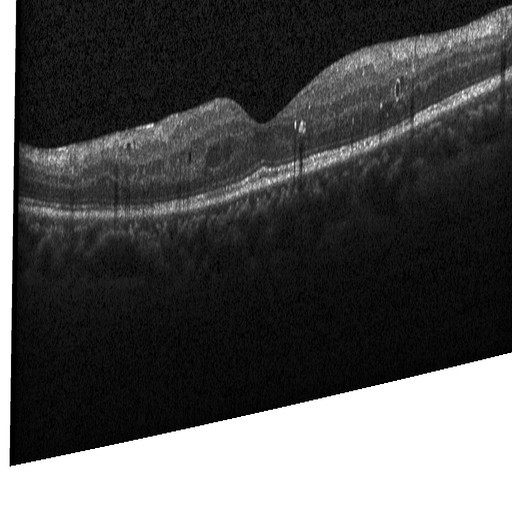

OCT scan showing diabetic macular edema.